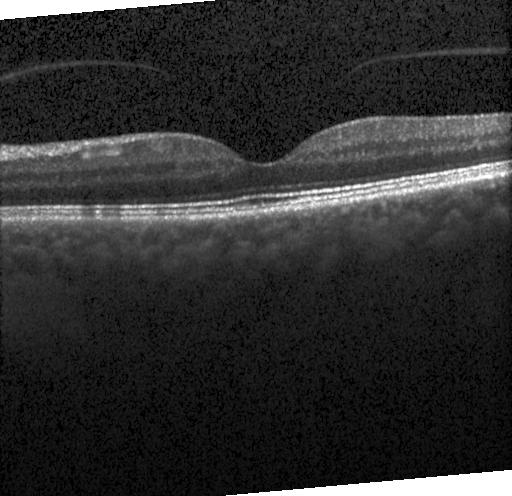
Centered on the fovea; optical coherence tomography scan; instrument: Heidelberg Spectralis — No evidence of choroidal neovascularization, diabetic macular edema, or drusen.